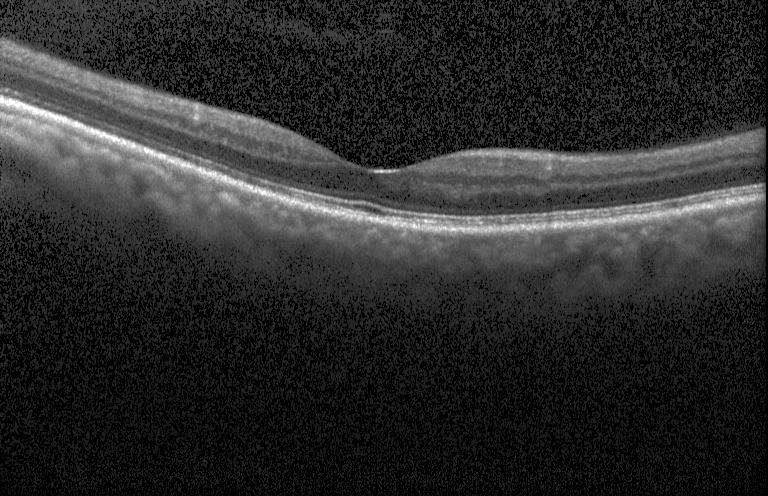
Heidelberg Spectralis OCT system; optical coherence tomography scan; spectral-domain OCT.
Finding: no evidence of choroidal neovascularization, diabetic macular edema, or drusen.